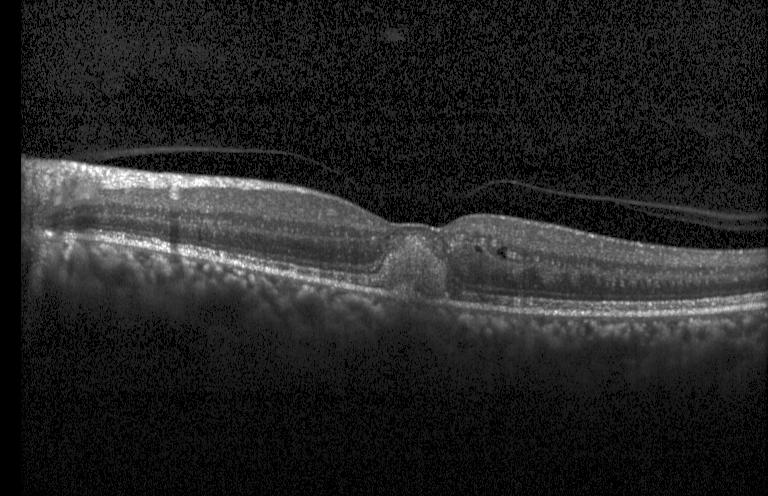 Optical coherence tomography scan.
Assessment: CNV.